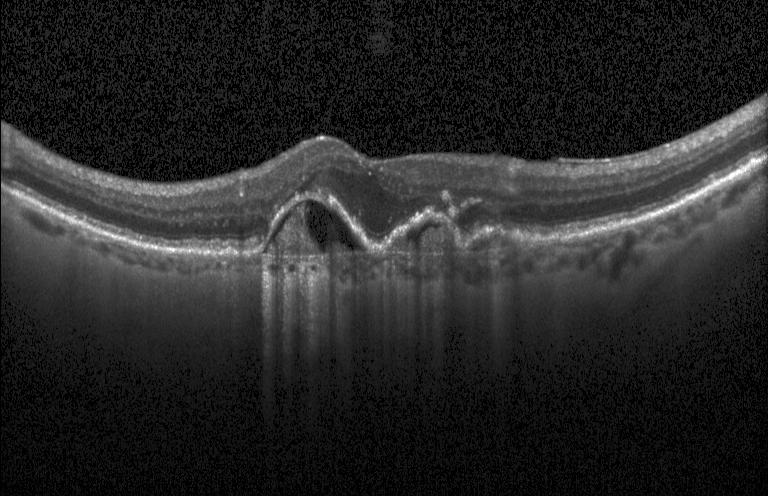

Heidelberg Spectralis. OCT B-scan. Spectral-domain OCT. Fovea-centered. Choroidal neovascularization (CNV).